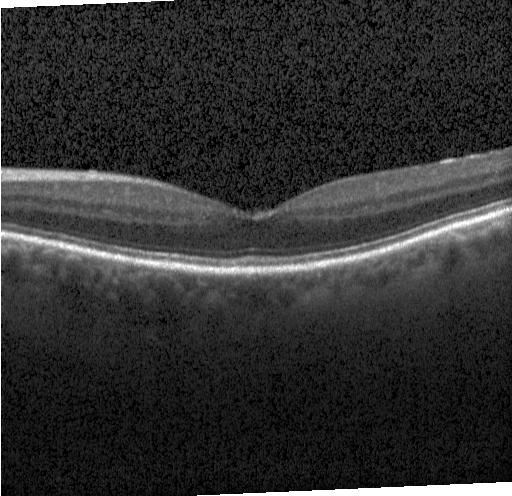
Finding: no choroidal neovascularization, diabetic macular edema, or drusen.